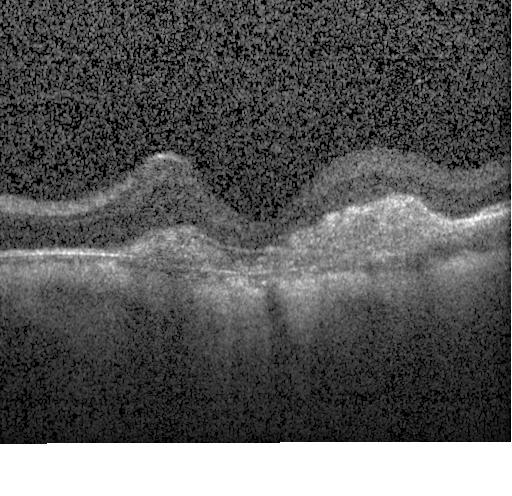
Retinal OCT B-scan, spectral-domain optical coherence tomography. The scan shows choroidal neovascularization.